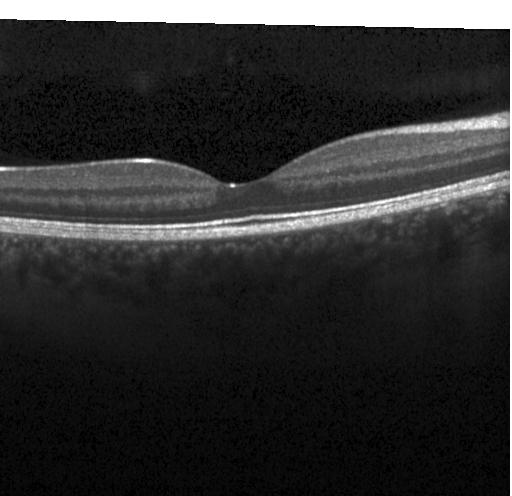

Macular OCT: neither choroidal neovascularization, diabetic macular edema, nor drusen.